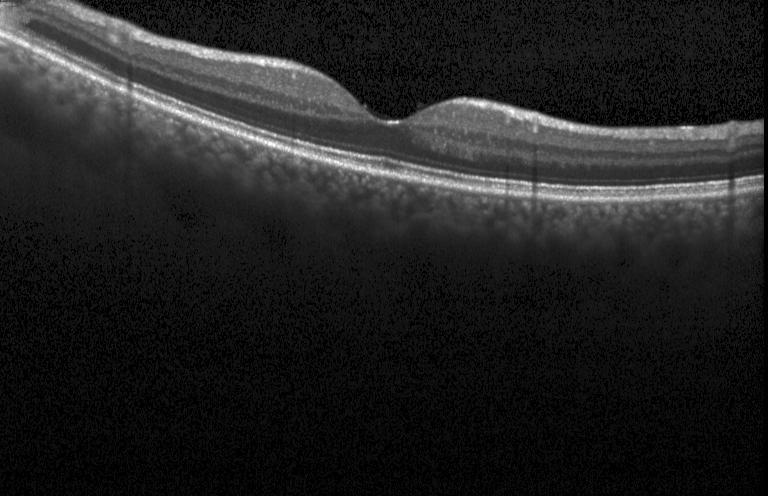 Retinal OCT B-scan.
This B-scan demonstrates no choroidal neovascularization, no diabetic macular edema, and no drusen.